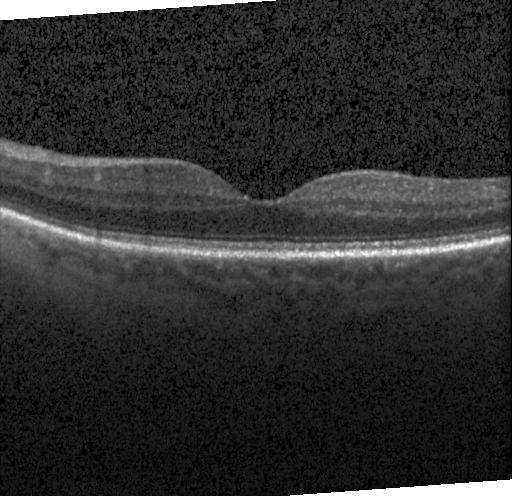
OCT finding: no evidence of choroidal neovascularization, diabetic macular edema, or drusen.